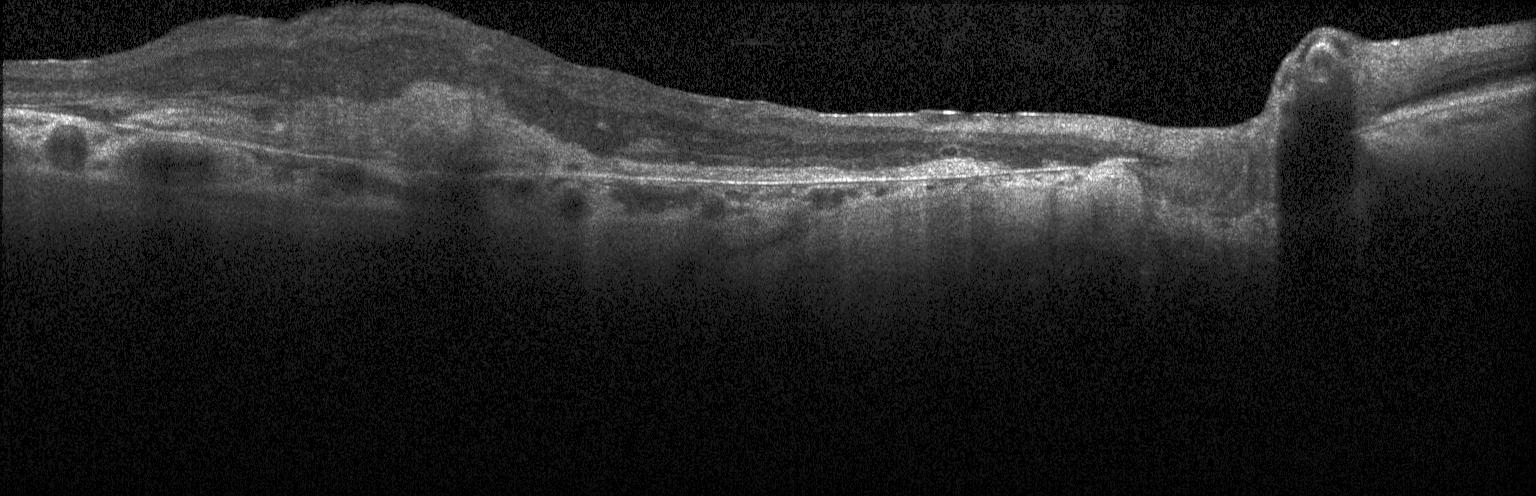 Choroidal neovascularization.